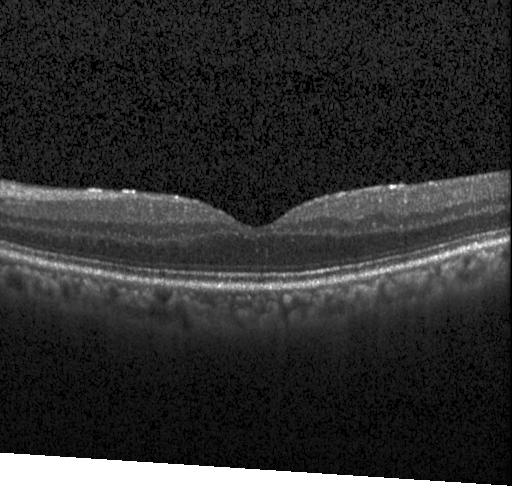

OCT B-scan; horizontal scan through the fovea.
Assessment: no CNV, DME, or drusen.